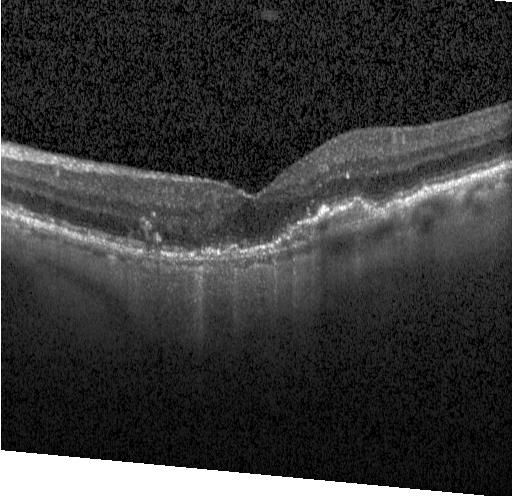
Finding: a choroidal neovascular membrane.